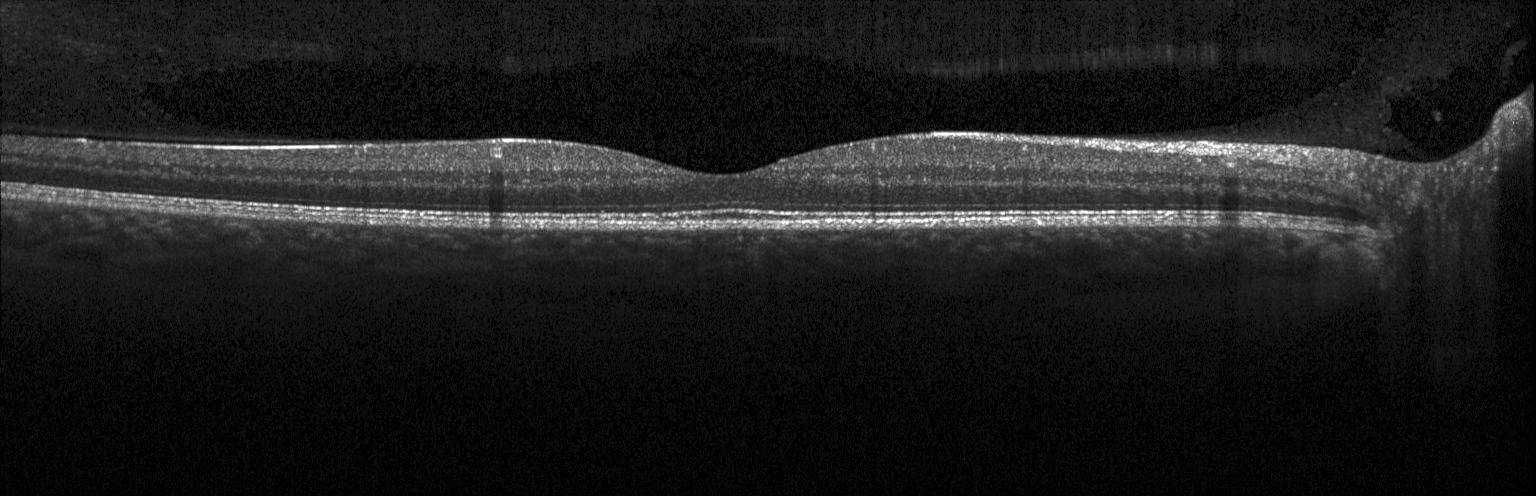

OCT B-scan. Instrument: Heidelberg Spectralis. Diagnosis: no choroidal neovascularization, no diabetic macular edema, and no drusen.